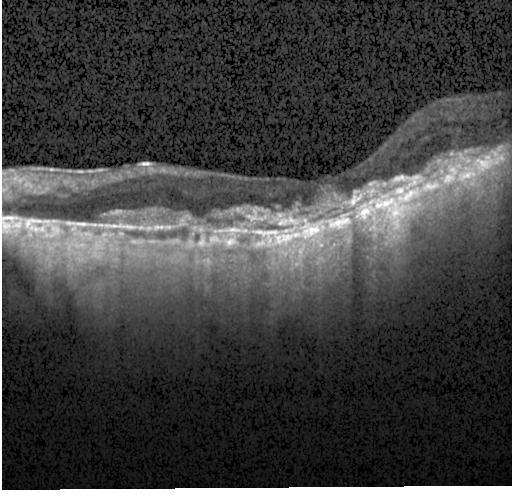 Macular OCT demonstrating a choroidal neovascular membrane.